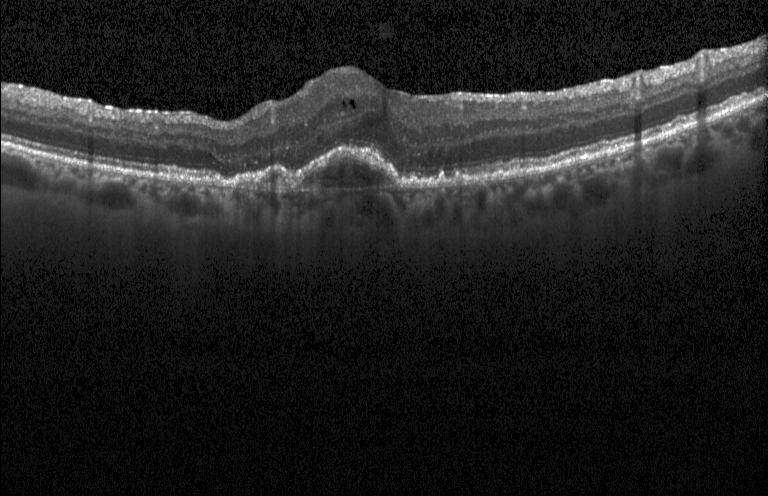
Retinal OCT cross-section showing a choroidal neovascular membrane.